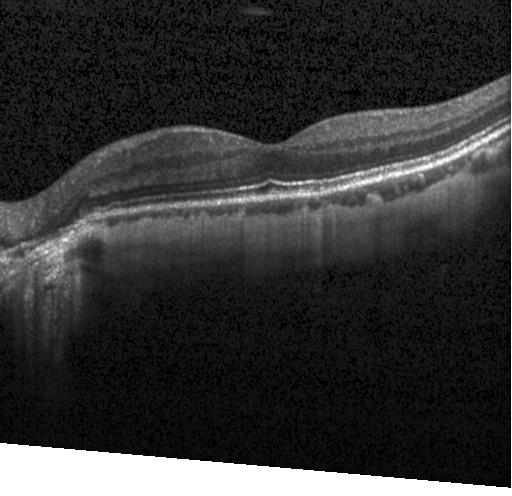
Centered on the fovea, acquired on a Heidelberg Spectralis, retinal OCT B-scan. Assessment: no choroidal neovascularization, no diabetic macular edema, and no drusen.